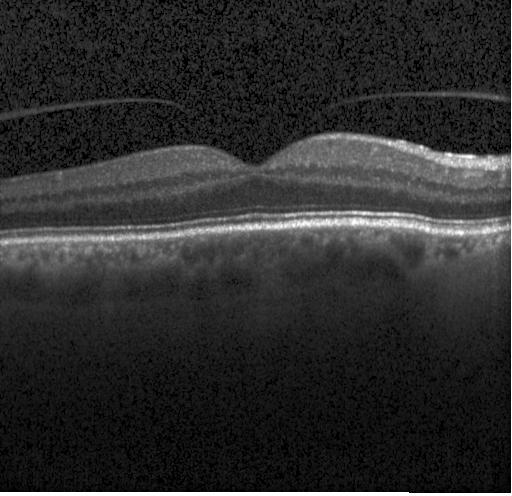
Retinal OCT B-scan · macular scan
Impression: neither CNV, DME, nor drusen.